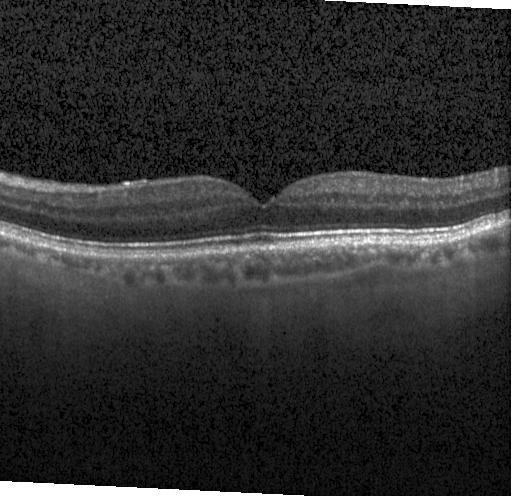

Optical coherence tomography B-scan. Spectral-domain OCT. Instrument: Heidelberg Spectralis. Centered on the fovea — Dx: no choroidal neovascularization, no diabetic macular edema, and no drusen.